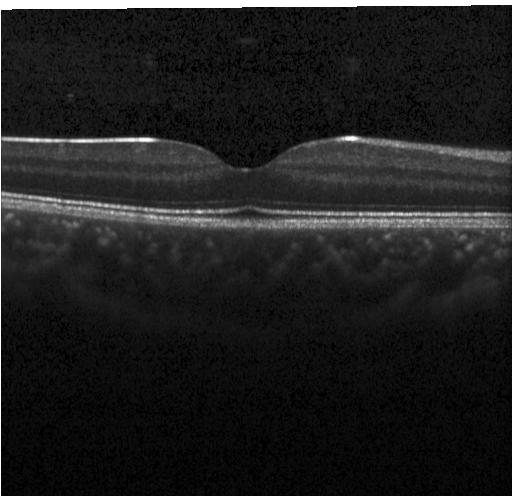

Centered on the fovea. Heidelberg Spectralis OCT system. Spectral-domain optical coherence tomography. OCT line scan
Impression: no evidence of choroidal neovascularization, diabetic macular edema, or drusen.